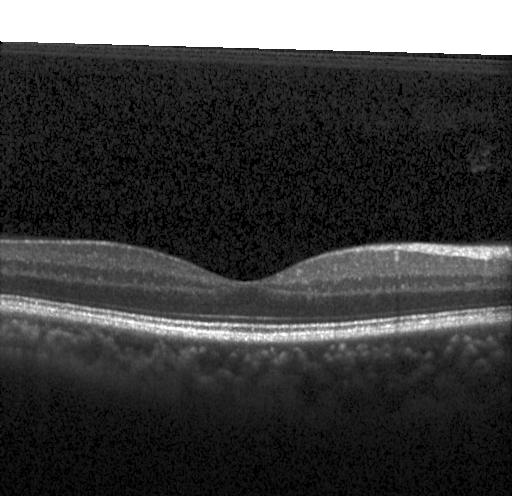

Heidelberg Spectralis OCT system. Through the macula. SD-OCT. OCT line scan — Dx: no CNV, no DME, and no drusen.